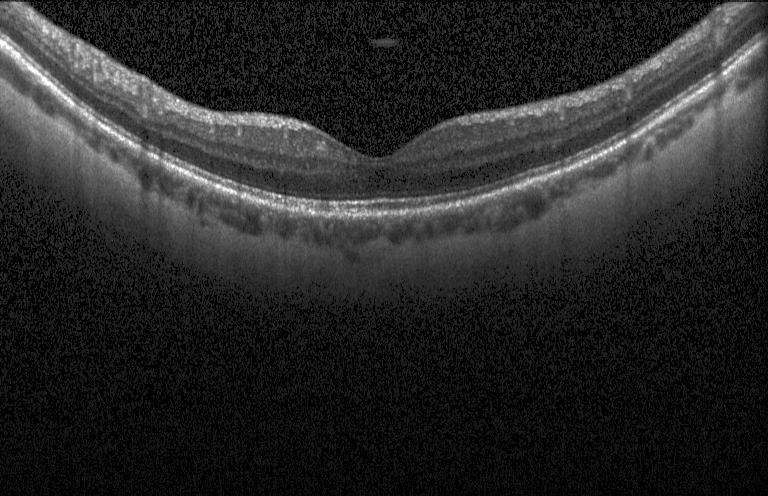 Assessment: neither CNV, DME, nor drusen.